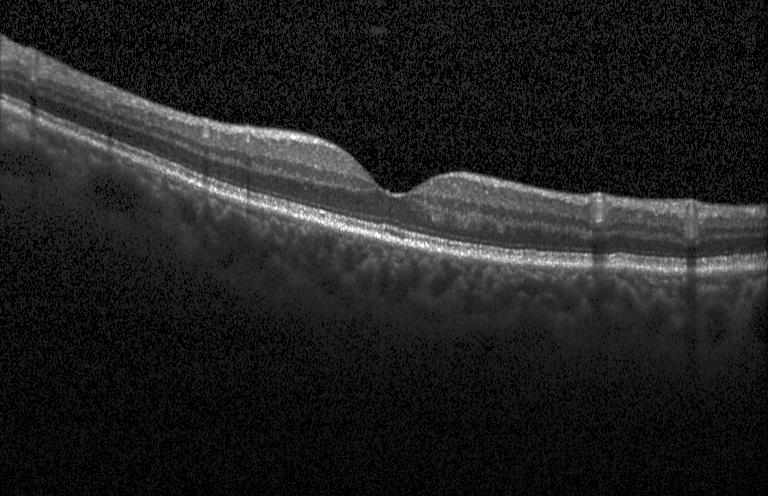
Centered on the fovea · OCT line scan · SD-OCT · Heidelberg Spectralis. Impression: no evidence of choroidal neovascularization, diabetic macular edema, or drusen.